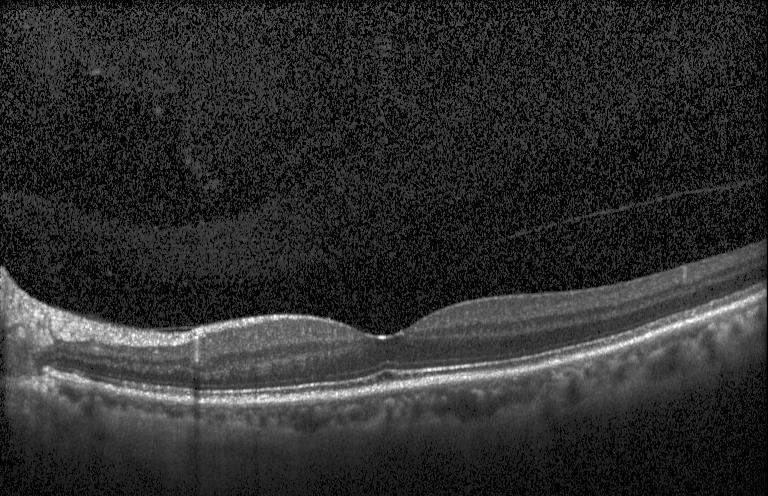
Retinal OCT B-scan; spectral-domain OCT; fovea-centered.
Assessment: no evidence of CNV, DME, or drusen.